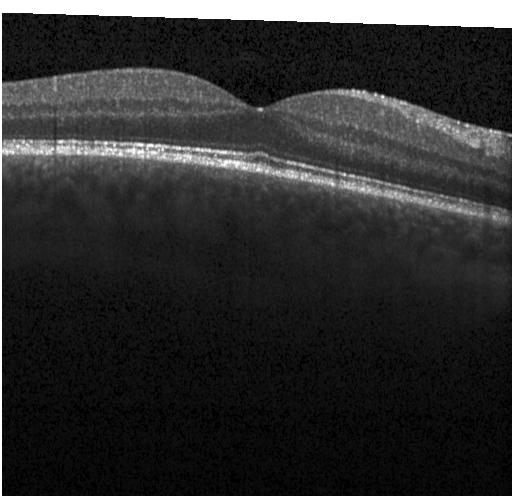
Horizontal scan through the fovea; spectral-domain optical coherence tomography; Heidelberg Spectralis OCT system; retinal OCT B-scan. Impression: no evidence of choroidal neovascularization, diabetic macular edema, or drusen.